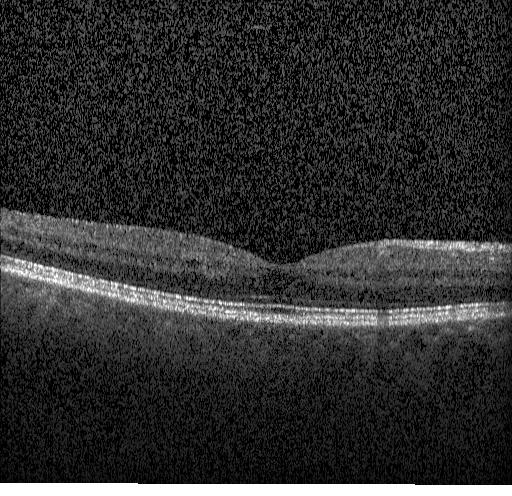
Optical coherence tomography scan; horizontal scan through the fovea
Dx: no evidence of choroidal neovascularization, diabetic macular edema, or drusen.